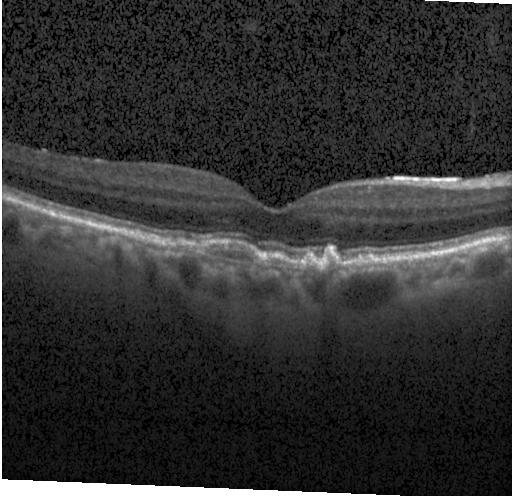 OCT B-scan — Impression: choroidal neovascularization (CNV).